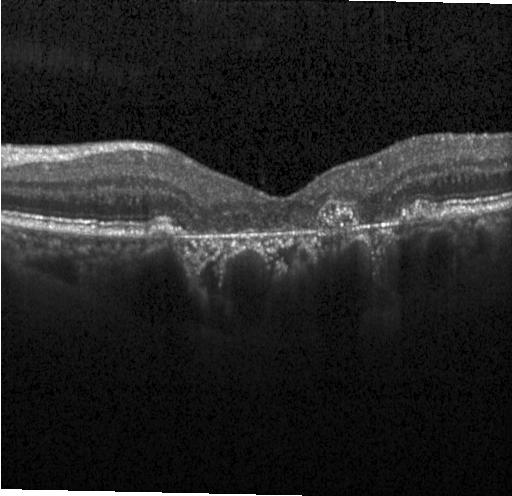 OCT B-scan showing a choroidal neovascular membrane.